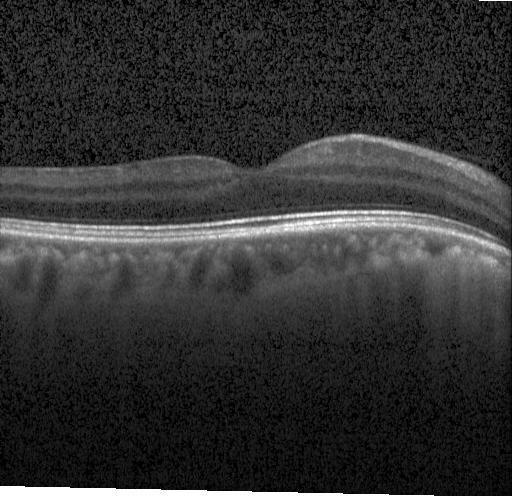 Retinal OCT cross-section
Assessment: neither choroidal neovascularization, diabetic macular edema, nor drusen.